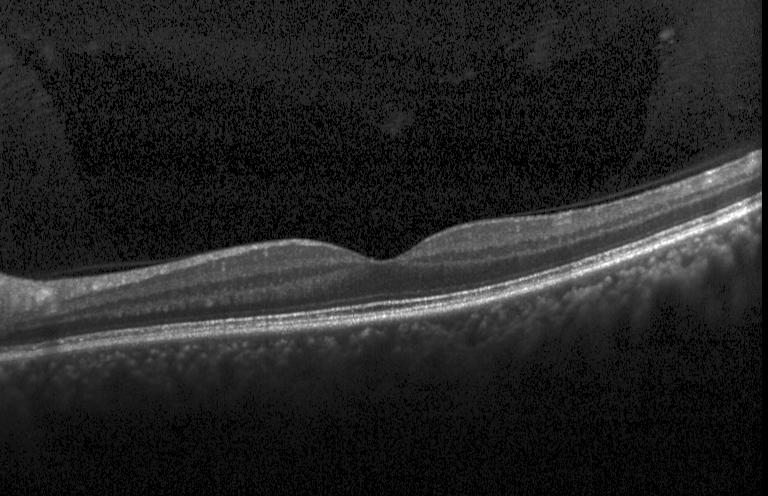 OCT line scan. Fovea-centered. Spectral-domain optical coherence tomography. Instrument: Heidelberg Spectralis. Diagnosis: neither CNV, DME, nor drusen.